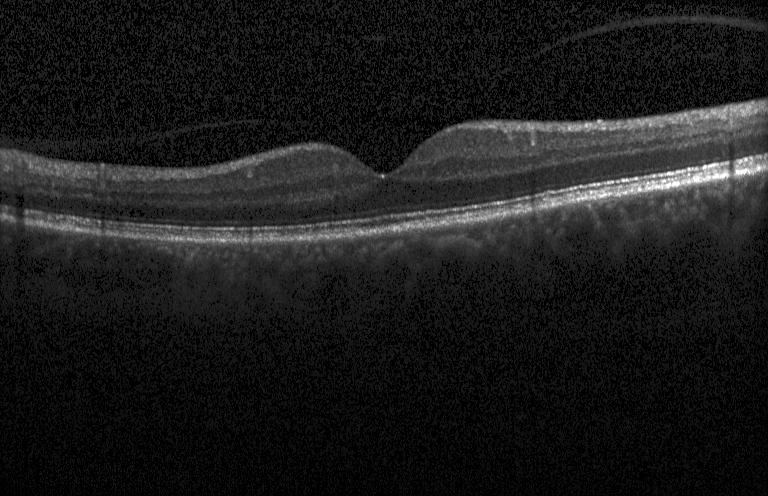

Optical coherence tomography scan; through the macula; acquired on a Heidelberg Spectralis; spectral-domain OCT. Macular OCT: no choroidal neovascularization, no diabetic macular edema, and no drusen.